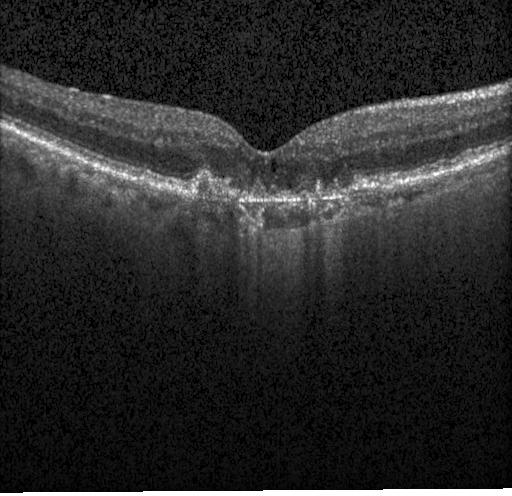 Optical coherence tomography B-scan
Impression: choroidal neovascularization (CNV).